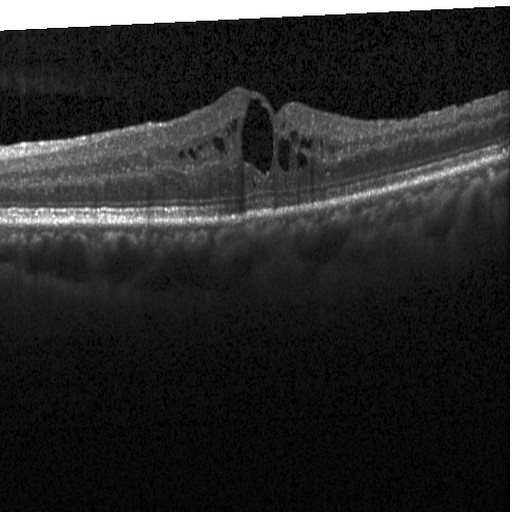 Optical coherence tomography scan. Impression: DME.